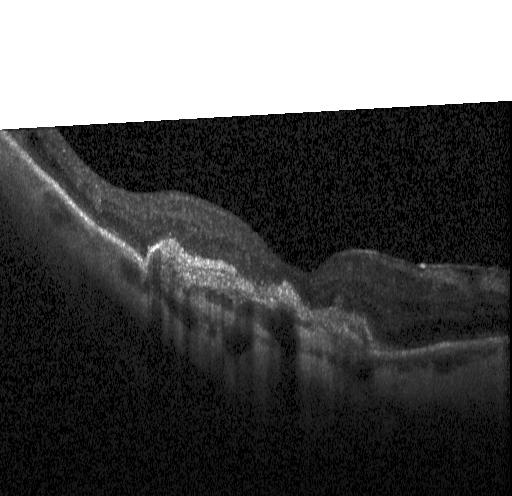

OCT line scan. Centered on the fovea. Spectral-domain optical coherence tomography
Impression: choroidal neovascularization (CNV).